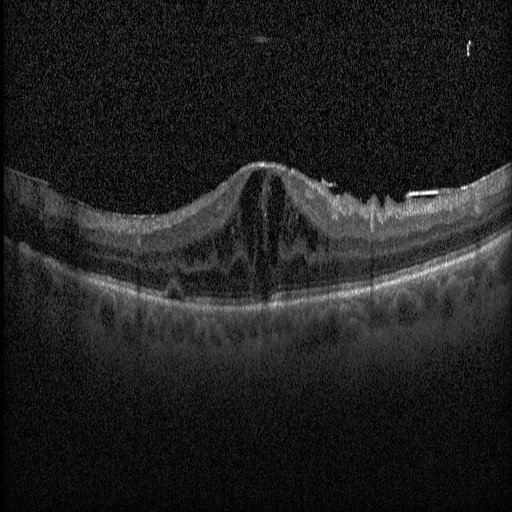 Impression: diabetic macular edema.